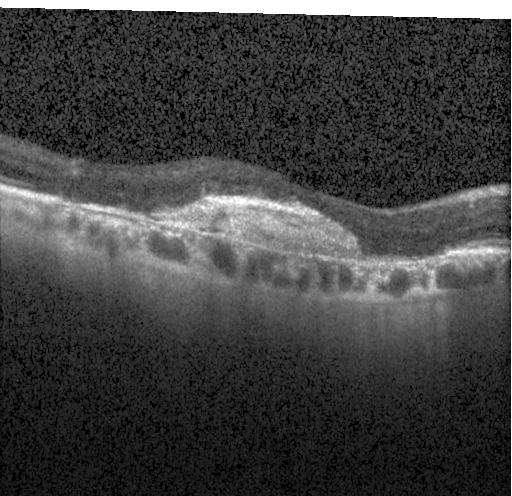

Fovea-centered. Optical coherence tomography B-scan. Heidelberg Spectralis. Spectral-domain OCT — Finding: a choroidal neovascular membrane.